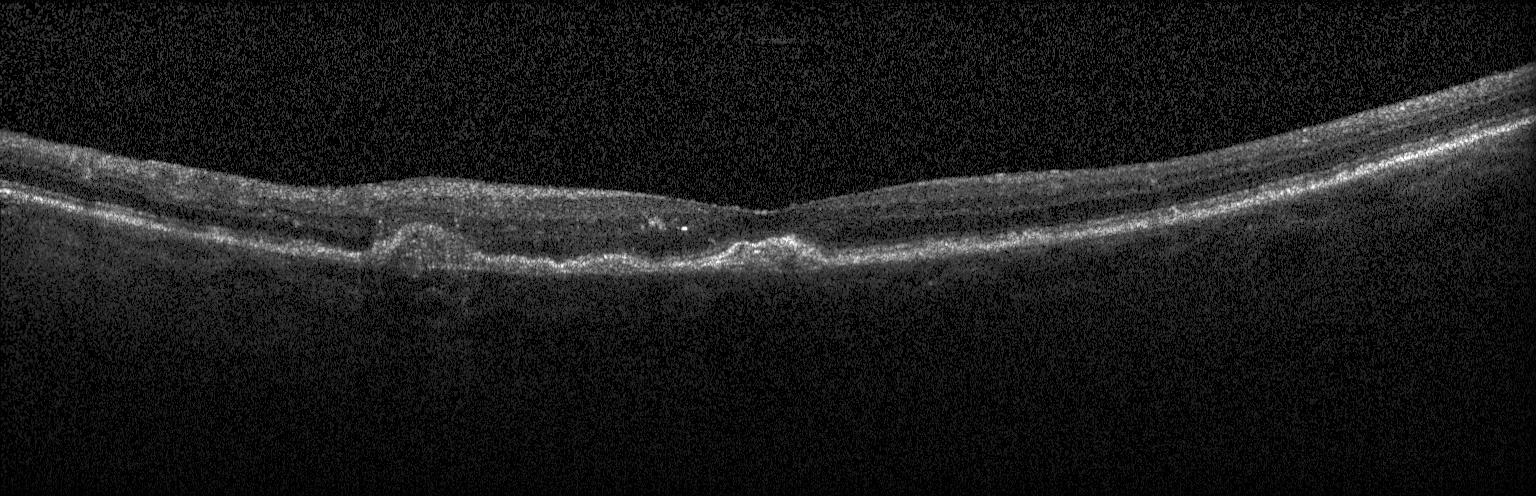 OCT finding: choroidal neovascularization (CNV).